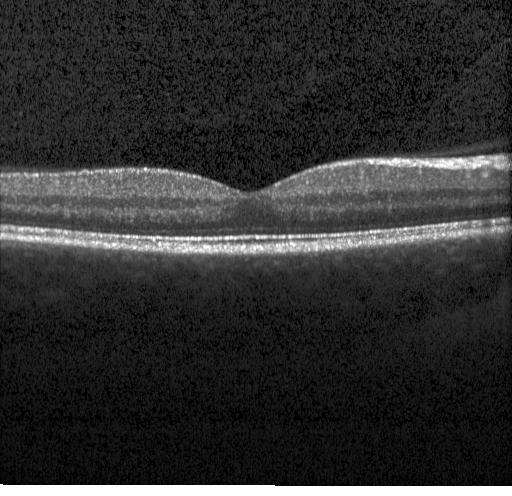

Optical coherence tomography B-scan. Through the macula. Spectral-domain OCT.
Impression: no CNV, no DME, and no drusen.